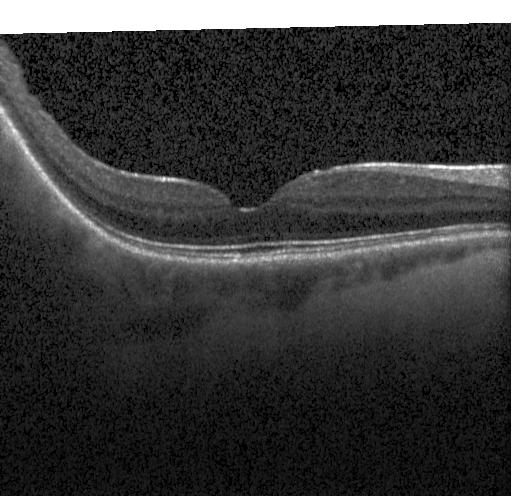

OCT B-scan.
Diagnosis: no choroidal neovascularization, no diabetic macular edema, and no drusen.